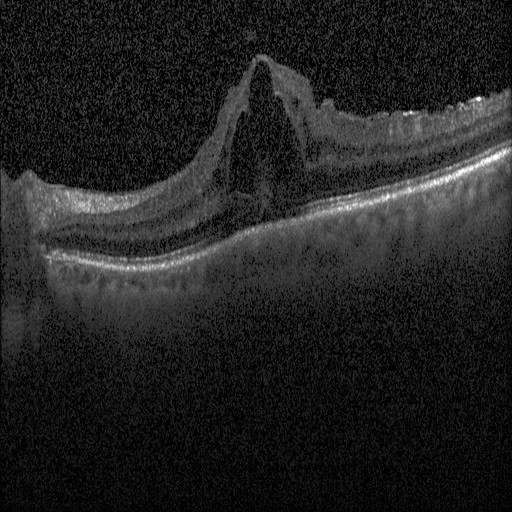 Horizontal scan through the fovea · optical coherence tomography B-scan · spectral-domain OCT · instrument: Heidelberg Spectralis — Diagnosis: diabetic macular edema (DME).